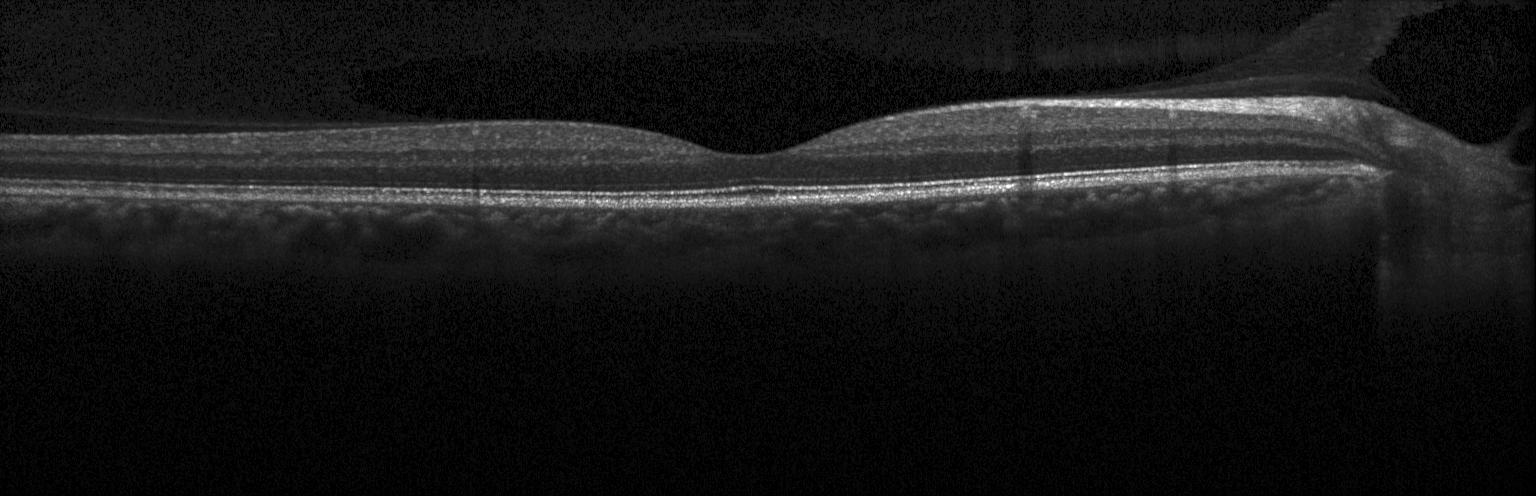

Optical coherence tomography B-scan; Heidelberg Spectralis OCT system. Macular OCT: no CNV, no DME, and no drusen.